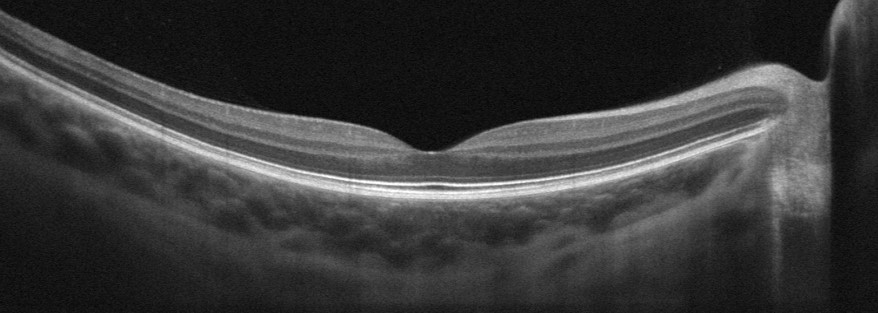 Retinal OCT cross-section. Fovea-centered.
Diagnosis: no AMD, DME, ERM, RAO, RVO, or VID.